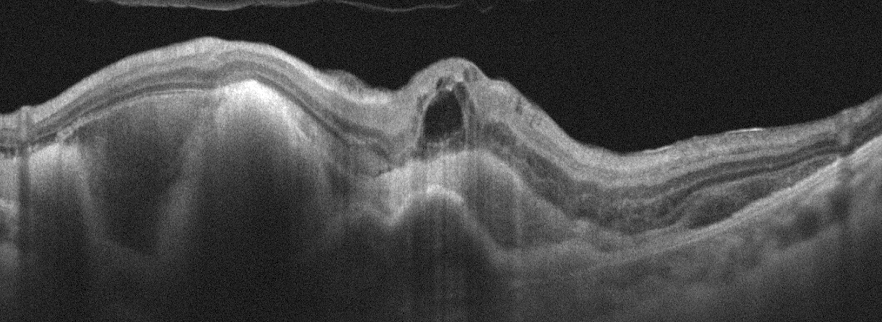
Dx: age-related macular degeneration (AMD).